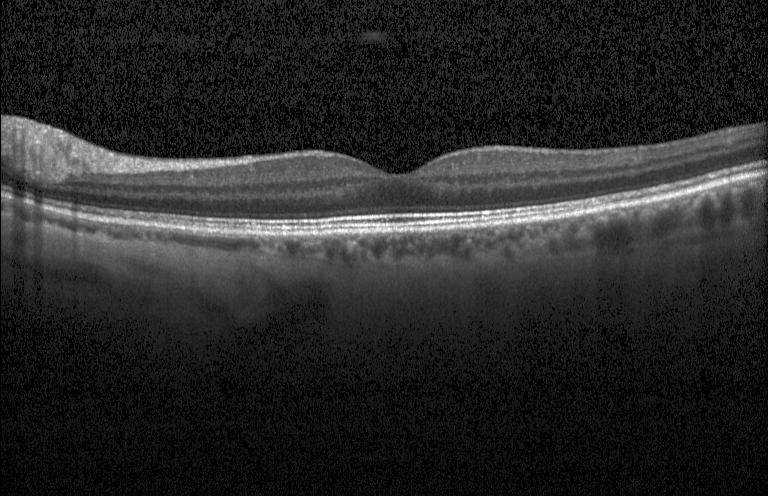 SD-OCT · OCT line scan · Heidelberg Spectralis OCT system · fovea-centered
Neither CNV, DME, nor drusen.